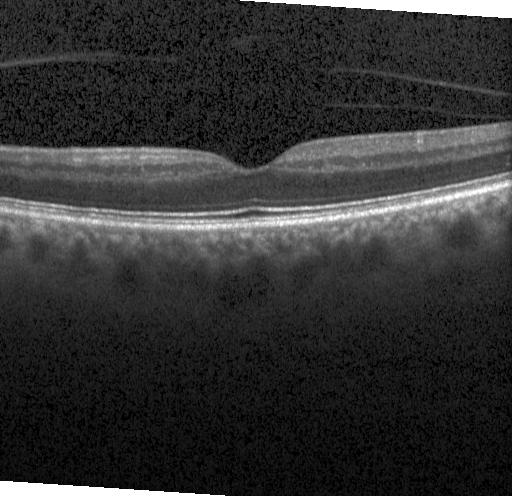 Macular scan; instrument: Heidelberg Spectralis; retinal OCT B-scan; SD-OCT — Assessment: no CNV, DME, or drusen.